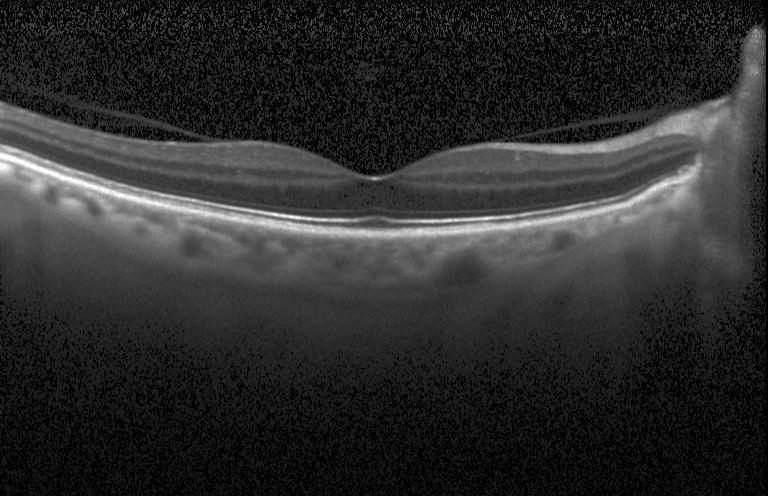

The scan shows no CNV, DME, or drusen.